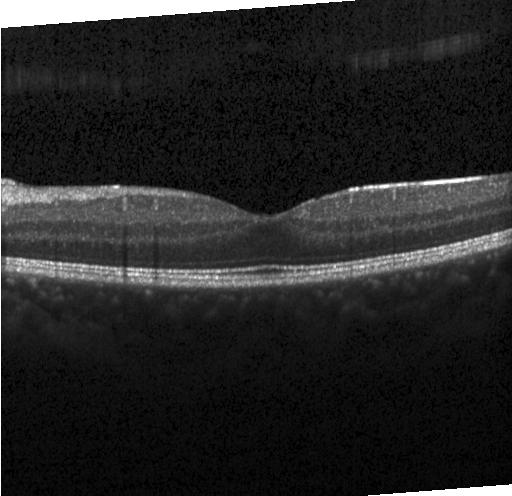 Spectral-domain OCT B-scan: no evidence of choroidal neovascularization, diabetic macular edema, or drusen.